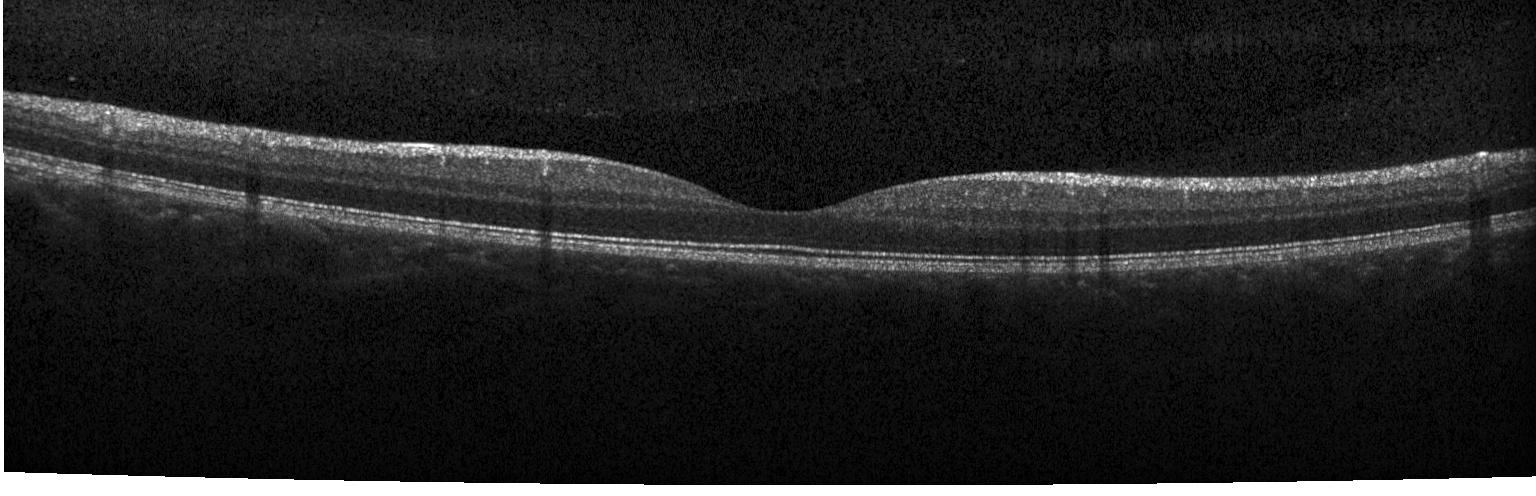

Assessment: no evidence of choroidal neovascularization, diabetic macular edema, or drusen.